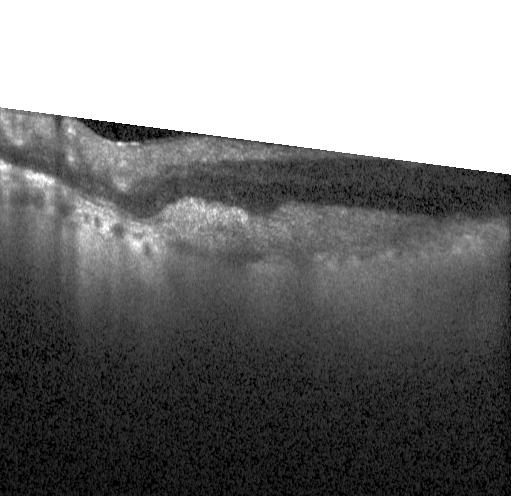
Macular scan. SD-OCT. OCT B-scan. Heidelberg Spectralis OCT system. Dx: a choroidal neovascular membrane.